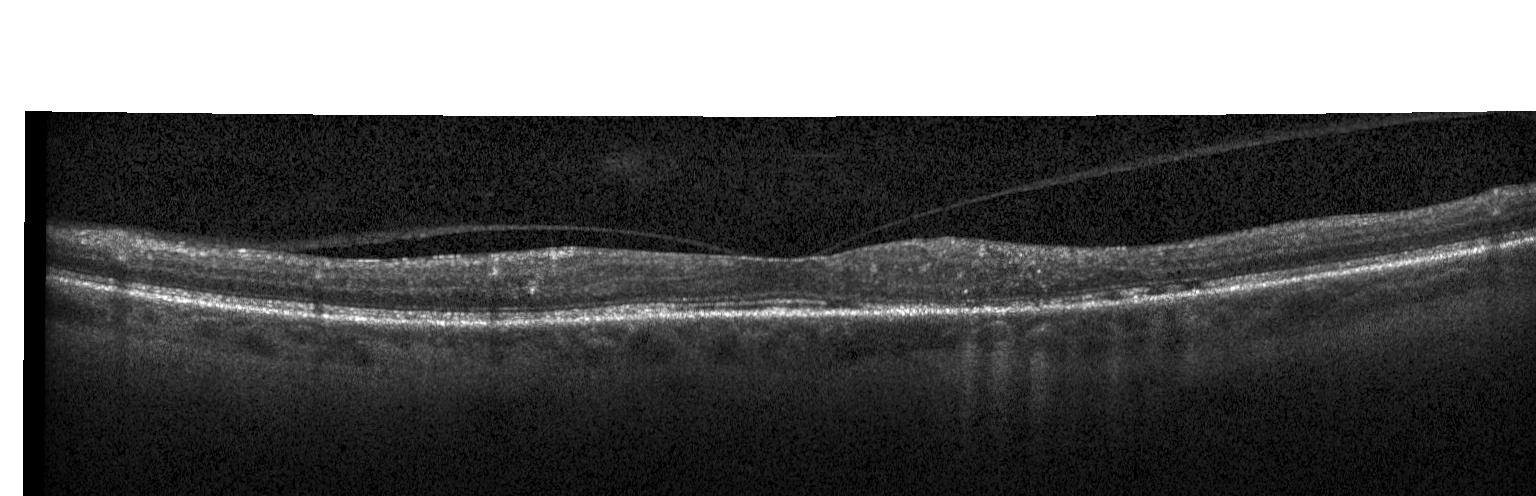 Fovea-centered · retinal OCT cross-section · spectral-domain optical coherence tomography · Heidelberg Spectralis OCT system. Impression: DME.